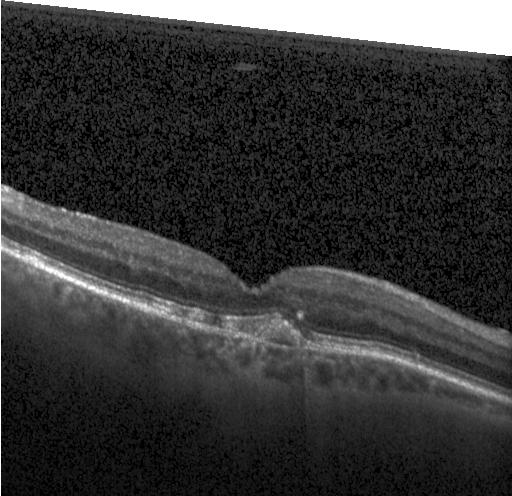
Retinal OCT cross-section showing CNV.